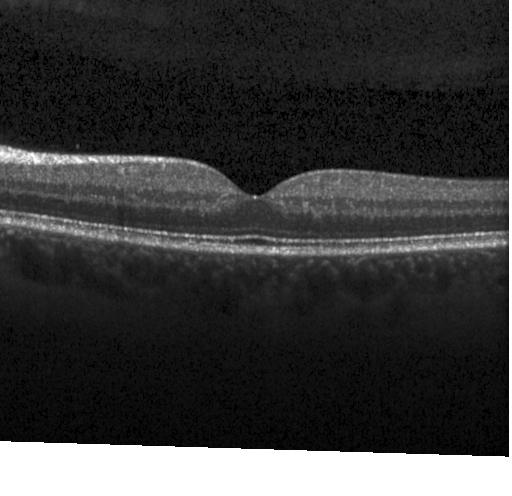
No CNV, no DME, and no drusen.